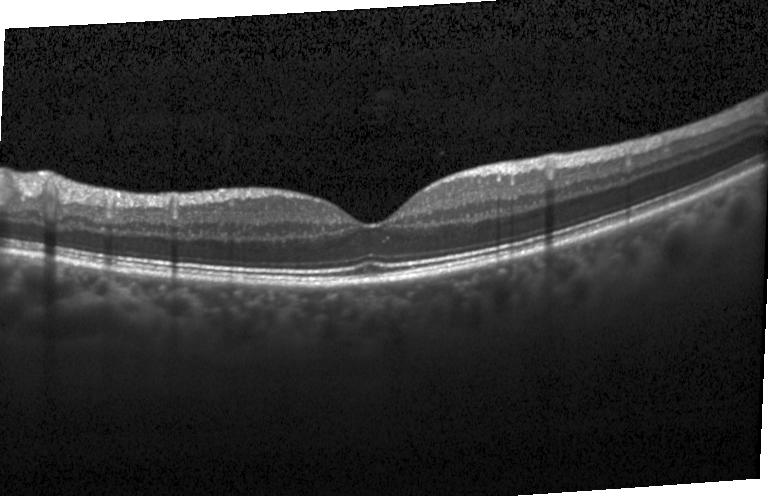

Finding: no CNV, DME, or drusen.